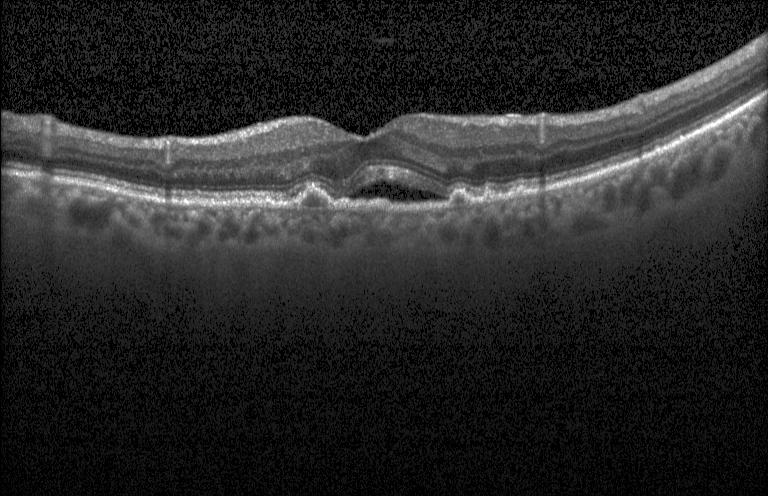
Dx: a choroidal neovascular membrane.